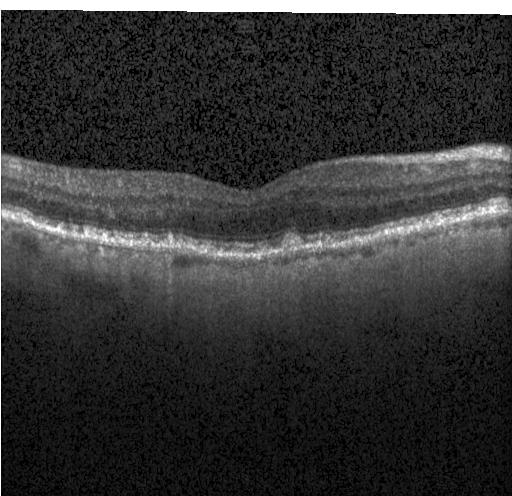

Assessment: multiple drusen.